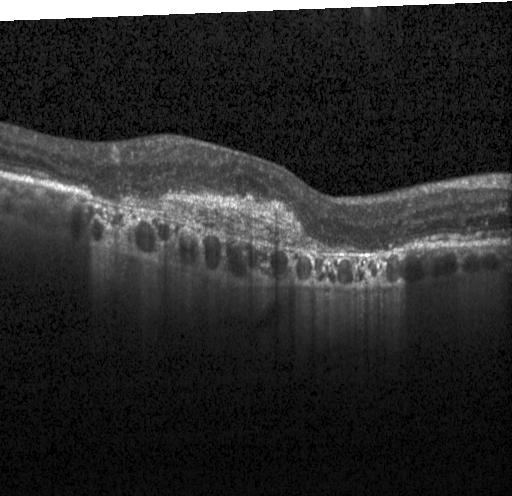

Through the macula. SD-OCT. Optical coherence tomography scan. Instrument: Heidelberg Spectralis. Macular OCT: a choroidal neovascular membrane.